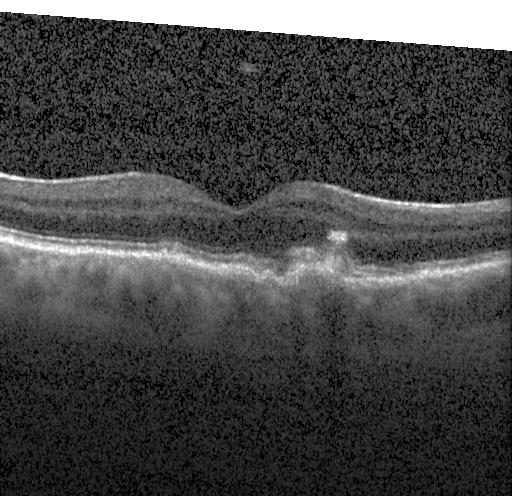

Dx: drusen.